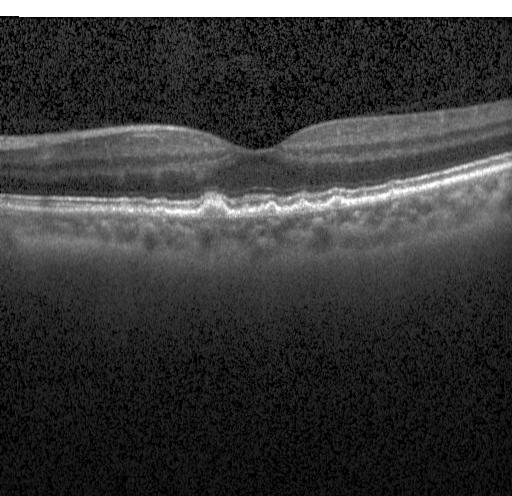
Optical coherence tomography B-scan, acquired on a Heidelberg Spectralis, horizontal scan through the fovea
Impression: drusen.